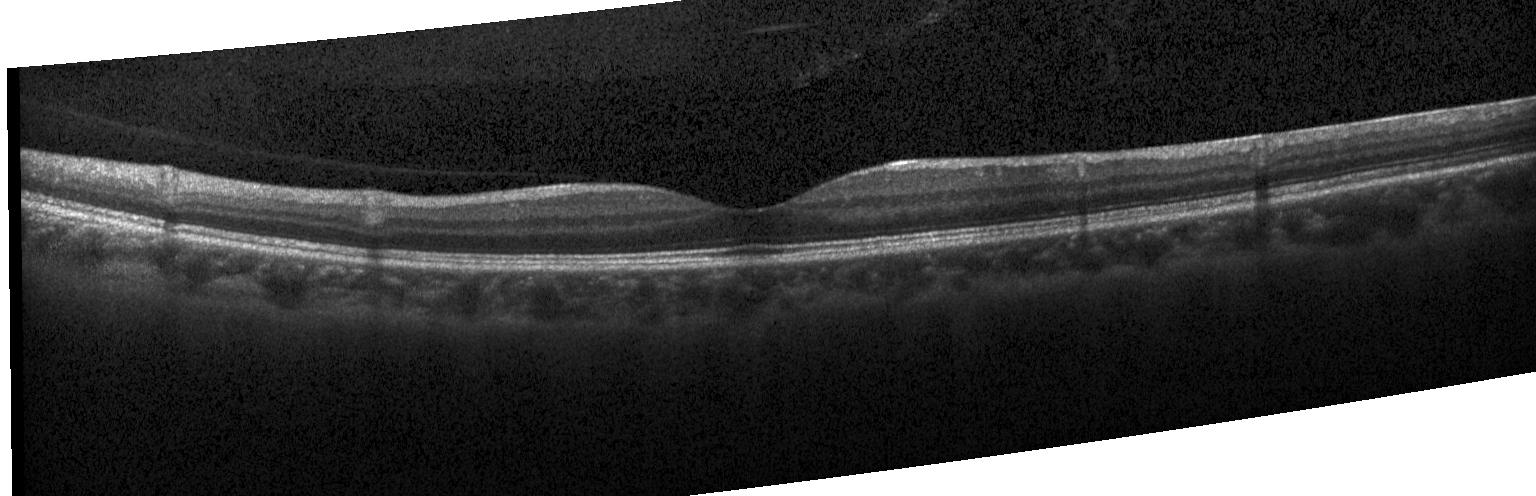
Heidelberg Spectralis · OCT B-scan.
Assessment: no evidence of choroidal neovascularization, diabetic macular edema, or drusen.